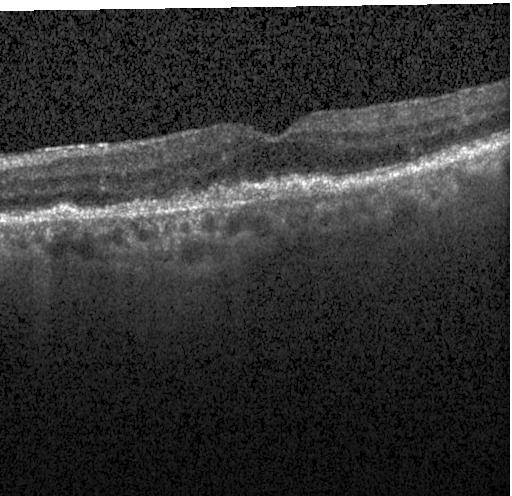 Retinal OCT cross-section showing choroidal neovascularization.